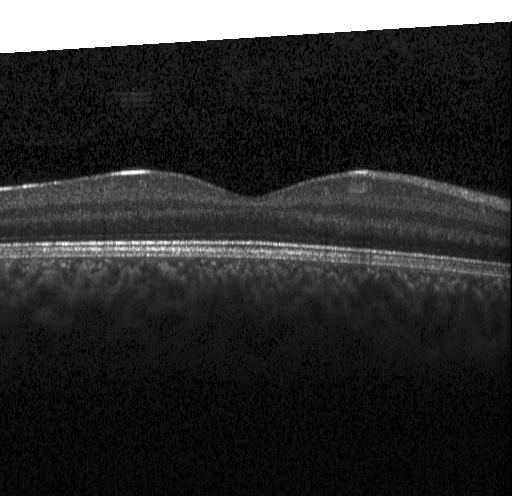 No evidence of choroidal neovascularization, diabetic macular edema, or drusen.